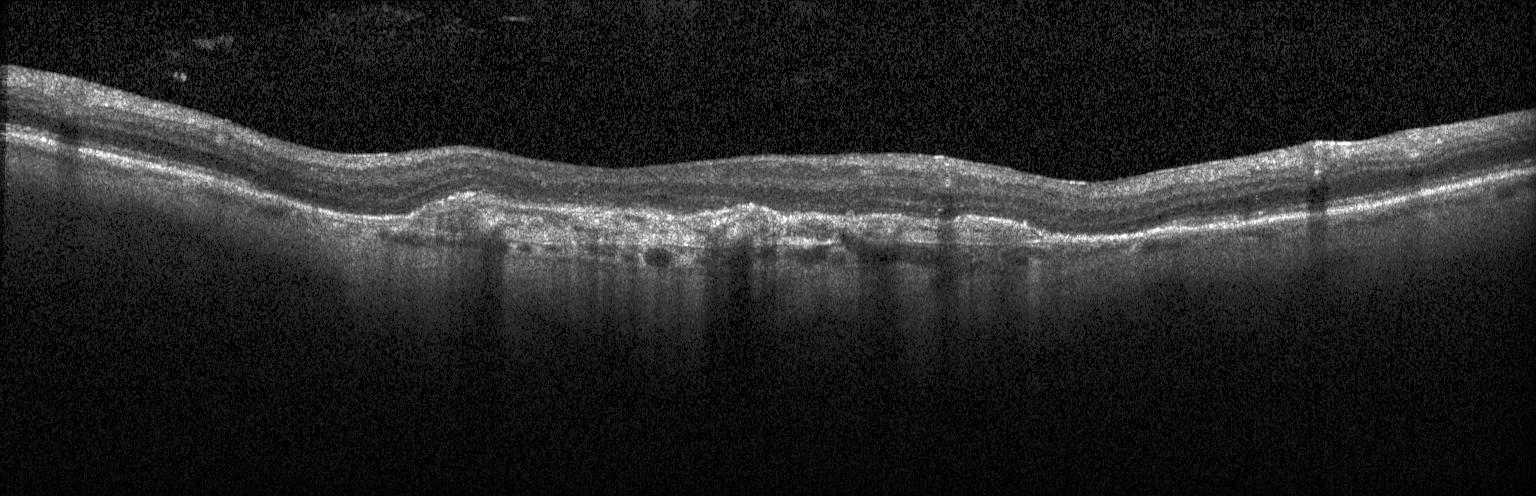

Macular OCT demonstrating CNV.